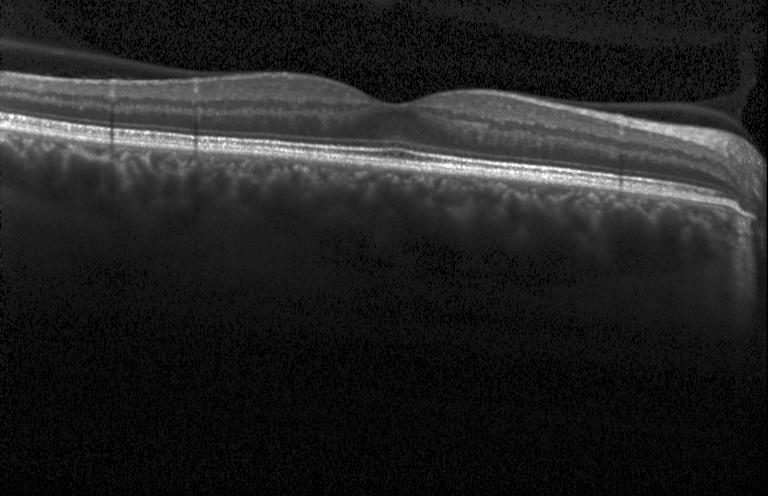

OCT B-scan showing no choroidal neovascularization, no diabetic macular edema, and no drusen.